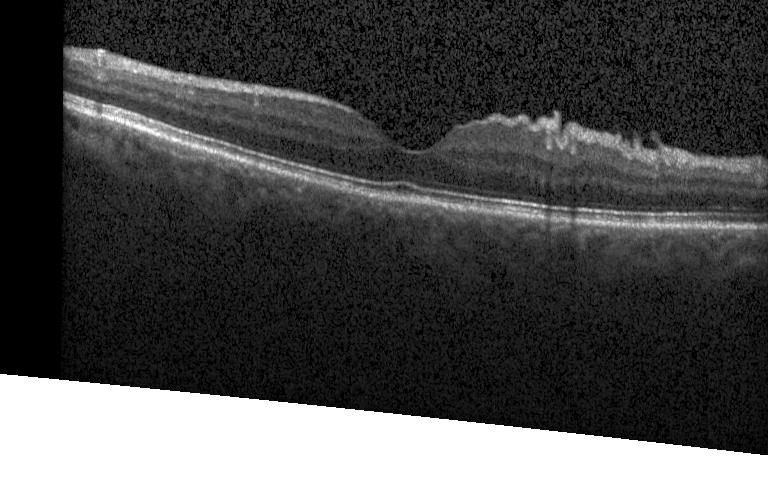
OCT line scan, SD-OCT — Diagnosis: no evidence of choroidal neovascularization, diabetic macular edema, or drusen.